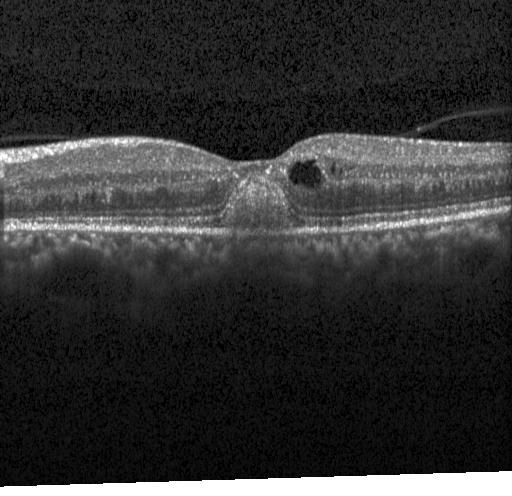
Centered on the fovea · retinal OCT cross-section · spectral-domain OCT — Diagnosis: choroidal neovascularization (CNV).